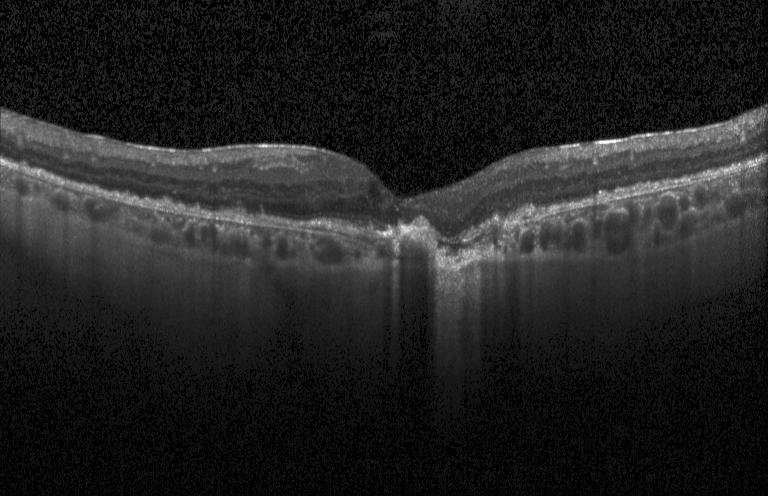 Optical coherence tomography scan. Macular scan. Instrument: Heidelberg Spectralis. The scan shows a choroidal neovascular membrane.